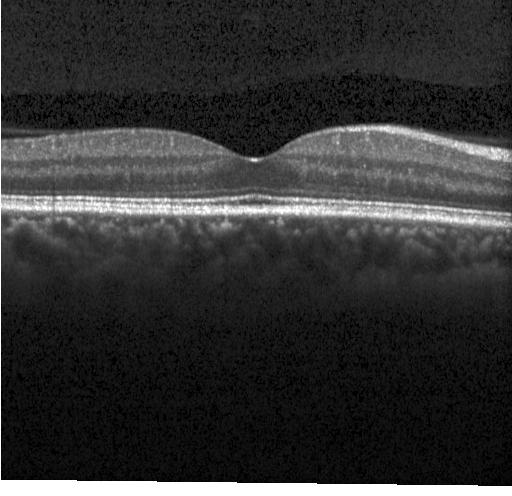
Retinal OCT cross-section showing neither choroidal neovascularization, diabetic macular edema, nor drusen.